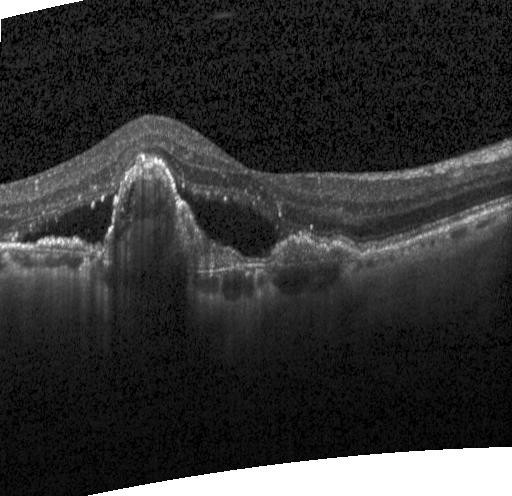 Retinal OCT B-scan · SD-OCT · centered on the fovea · acquired on a Heidelberg Spectralis
Impression: choroidal neovascularization.